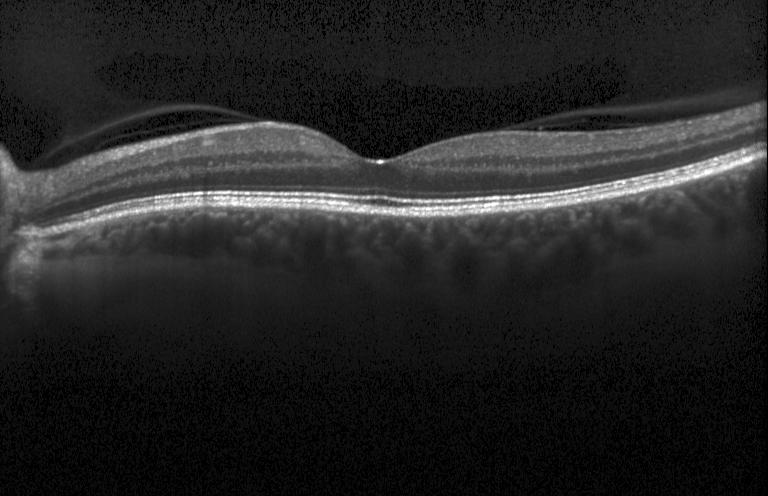
Finding: no choroidal neovascularization, no diabetic macular edema, and no drusen.